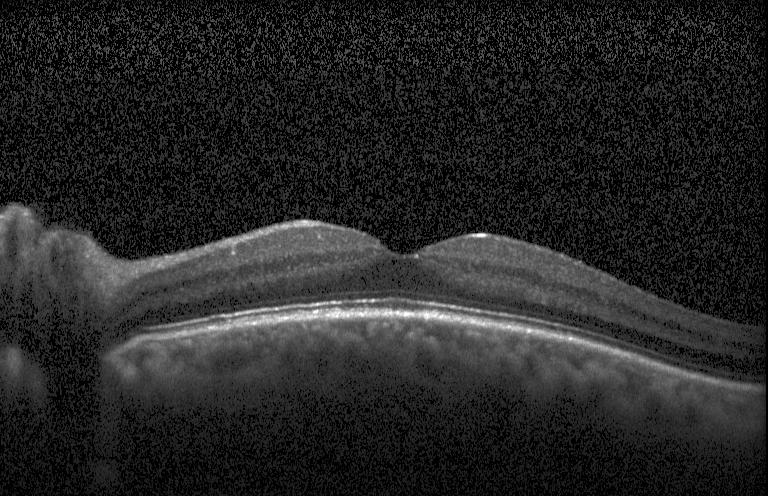 Impression: neither choroidal neovascularization, diabetic macular edema, nor drusen.